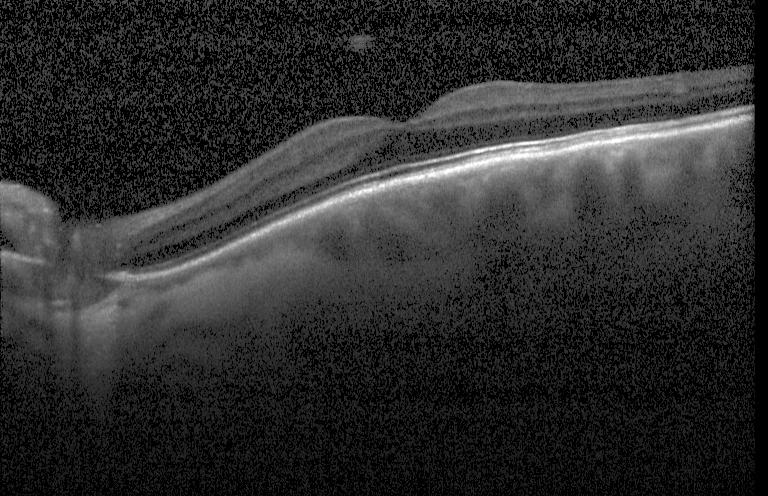
Retinal OCT cross-section showing no evidence of CNV, DME, or drusen.